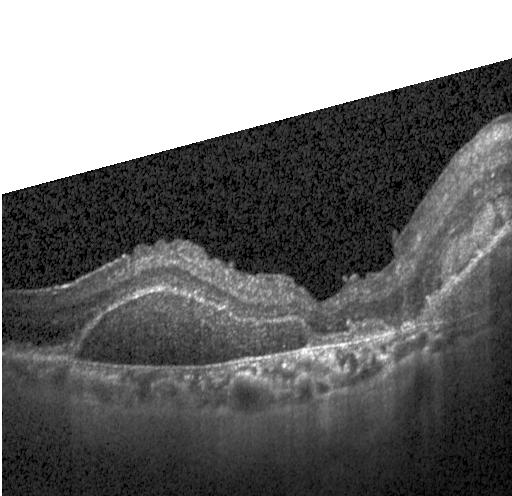

Finding: choroidal neovascularization.